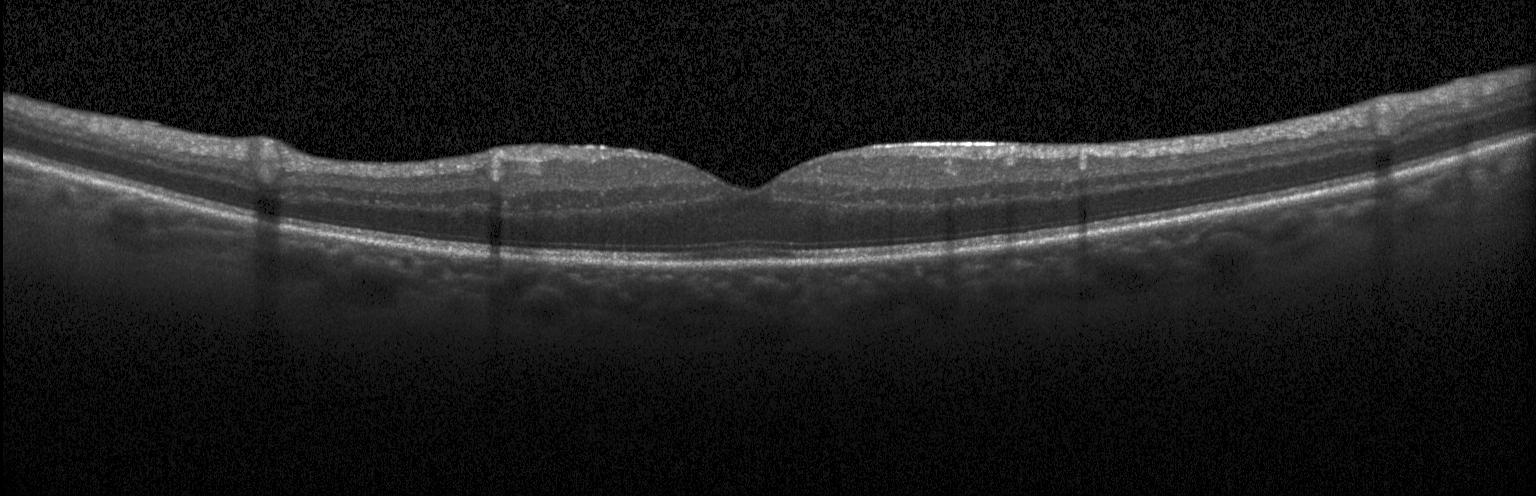
Diagnosis: neither choroidal neovascularization, diabetic macular edema, nor drusen.